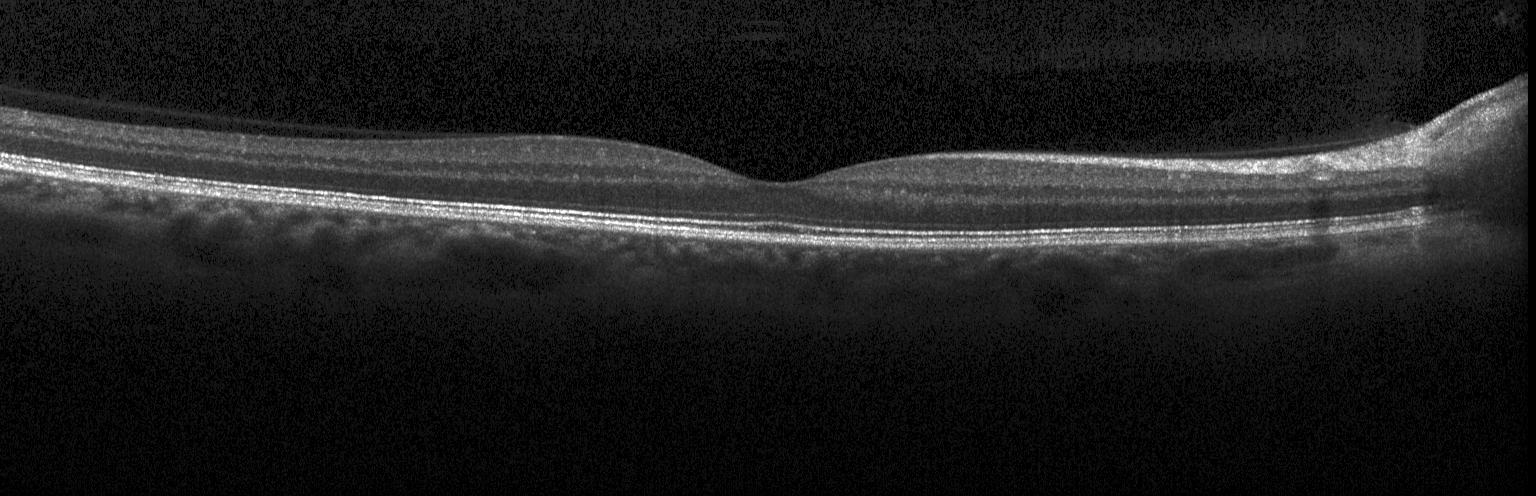
Spectral-domain OCT B-scan: no CNV, DME, or drusen.